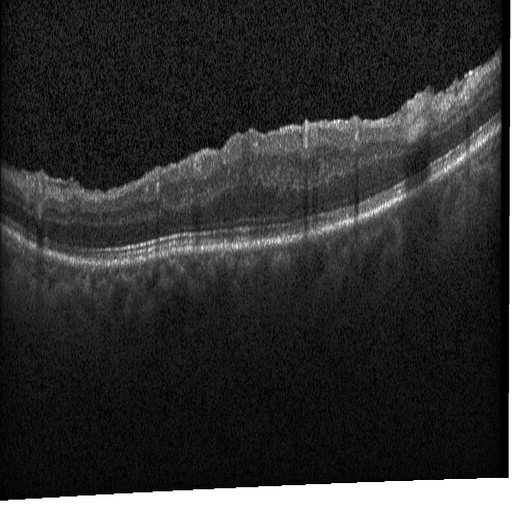

Diabetic macular edema (DME).